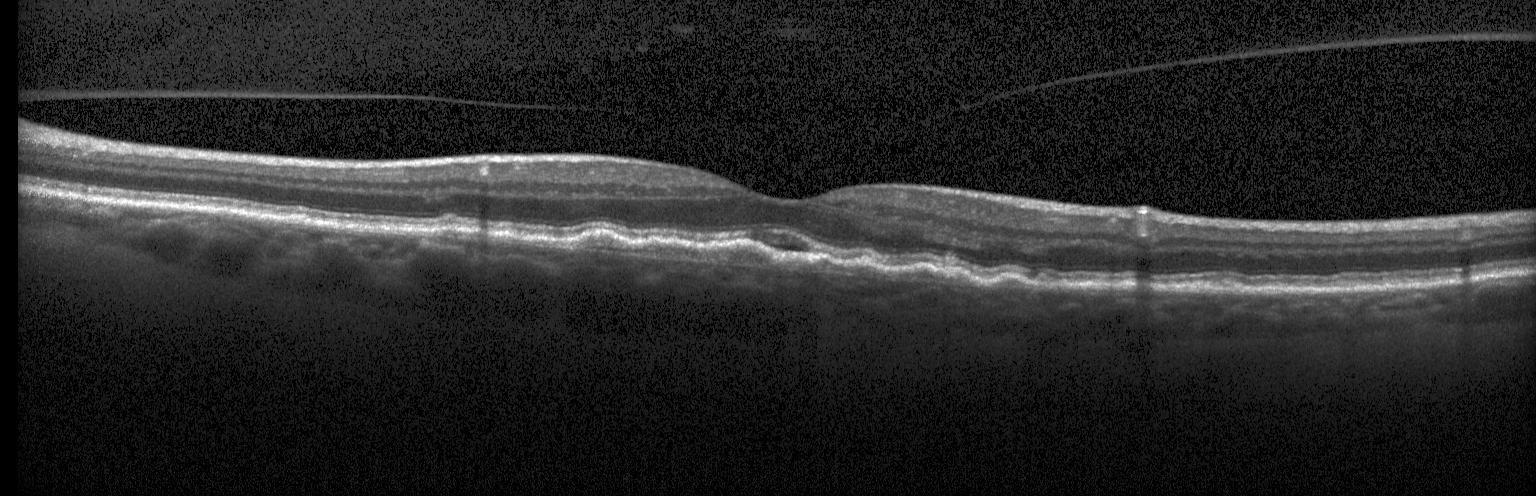

OCT finding: a choroidal neovascular membrane.